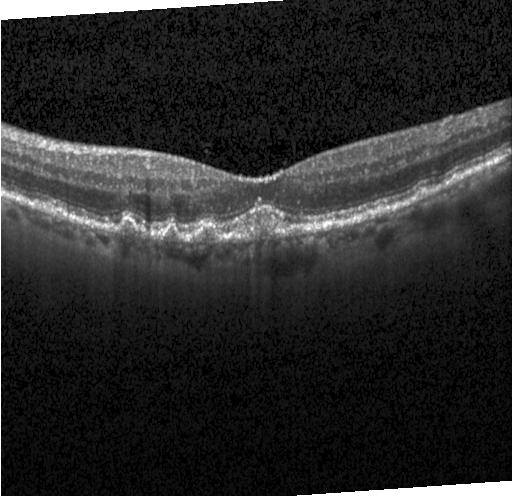
Dx: drusen.